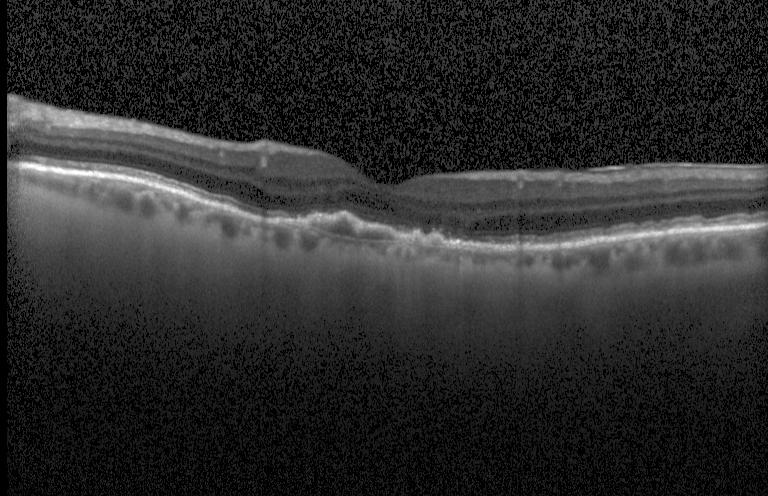 Diagnosis: choroidal neovascularization (CNV).